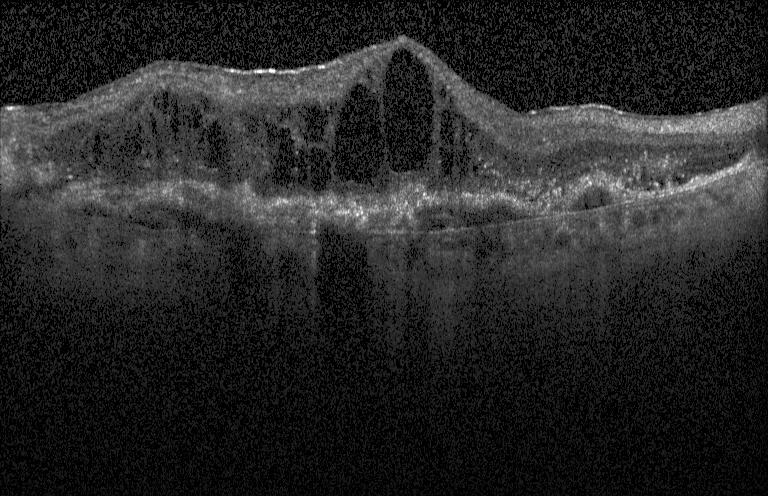

Retinal OCT cross-section showing a choroidal neovascular membrane.